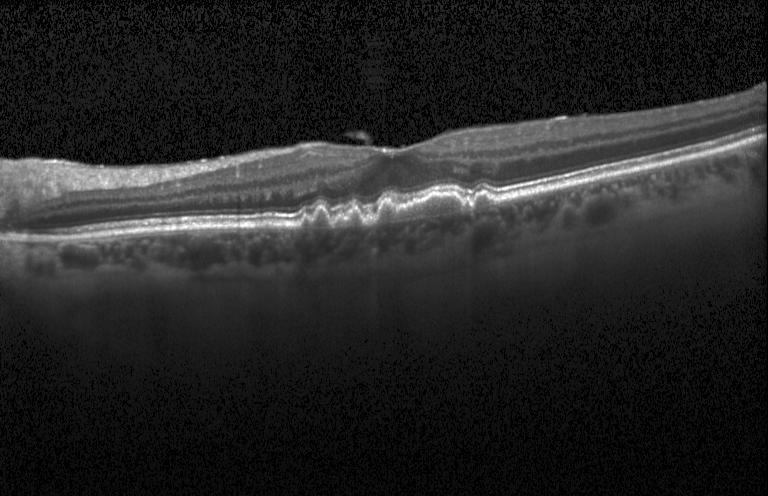 OCT scan showing sub-RPE drusenoid deposits.